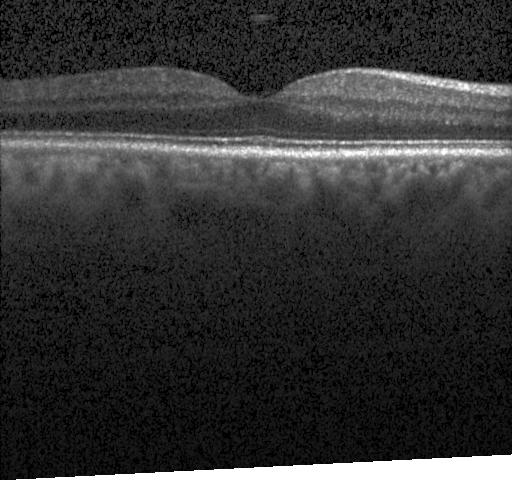
Assessment: no choroidal neovascularization, no diabetic macular edema, and no drusen.